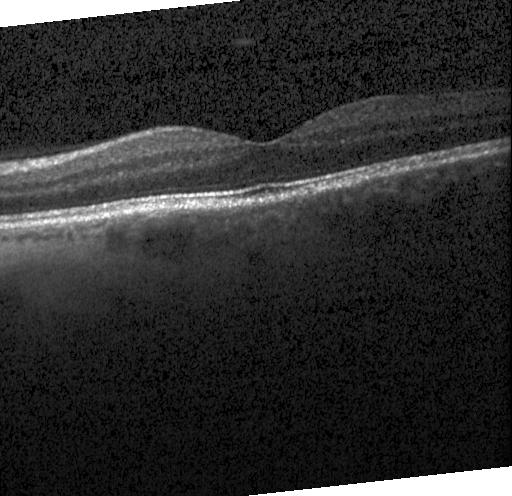

Finding: no evidence of choroidal neovascularization, diabetic macular edema, or drusen.